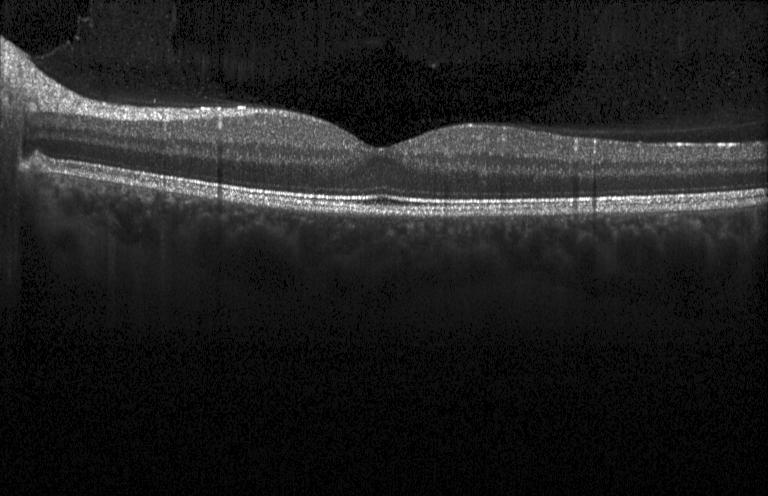 Instrument: Heidelberg Spectralis · retinal OCT cross-section · horizontal scan through the fovea — Assessment: neither CNV, DME, nor drusen.